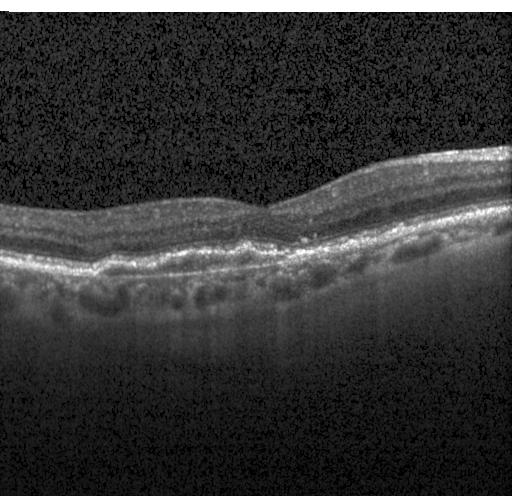
Optical coherence tomography scan, centered on the fovea, acquired on a Heidelberg Spectralis, spectral-domain optical coherence tomography.
Finding: a choroidal neovascular membrane.